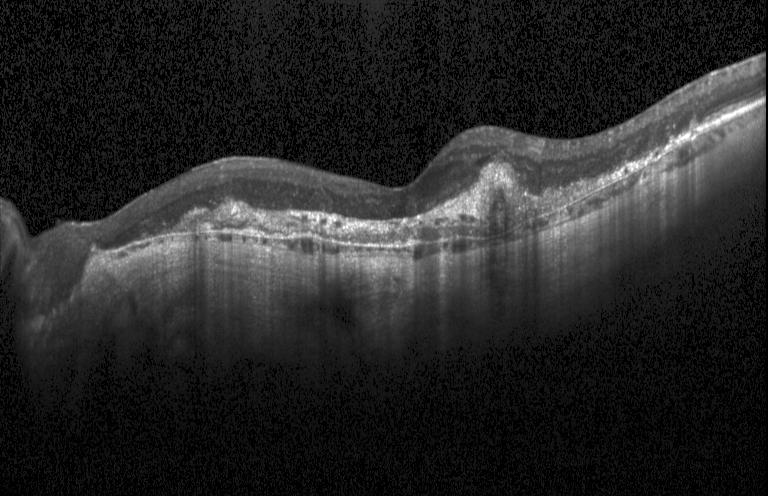 Retinal OCT cross-section showing a choroidal neovascular membrane.